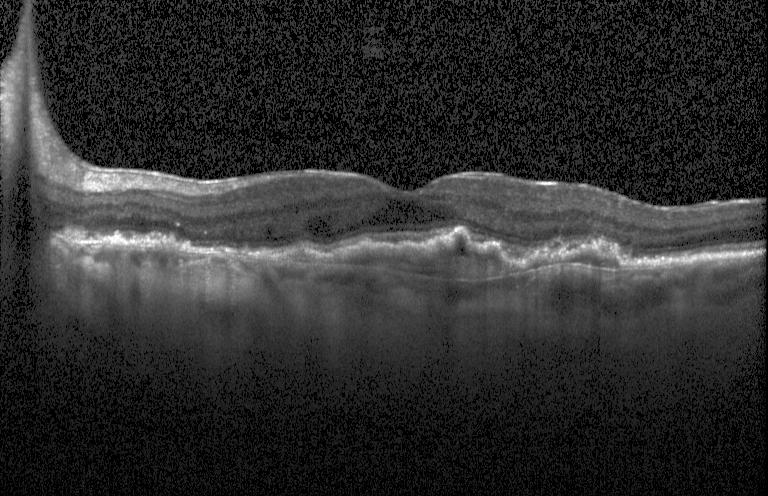

Diagnosis: a choroidal neovascular membrane.